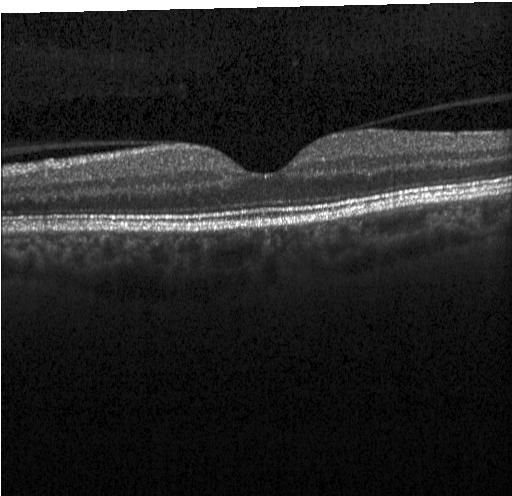
Optical coherence tomography B-scan. Diagnosis: no evidence of choroidal neovascularization, diabetic macular edema, or drusen.